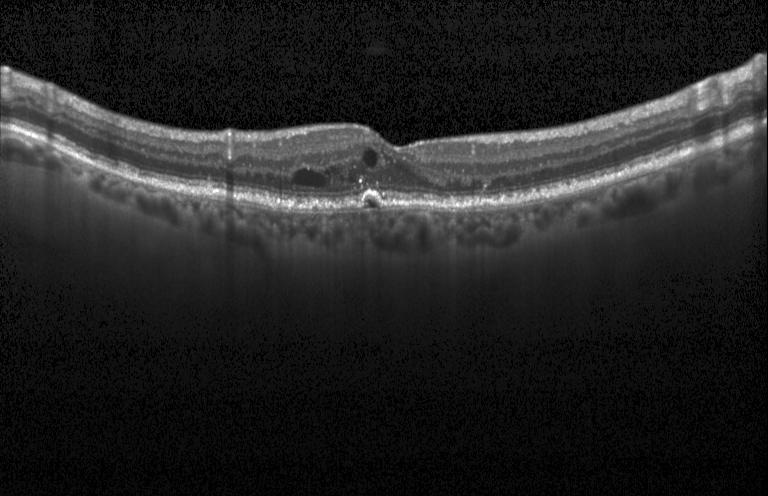 Retinal OCT B-scan. A choroidal neovascular membrane.